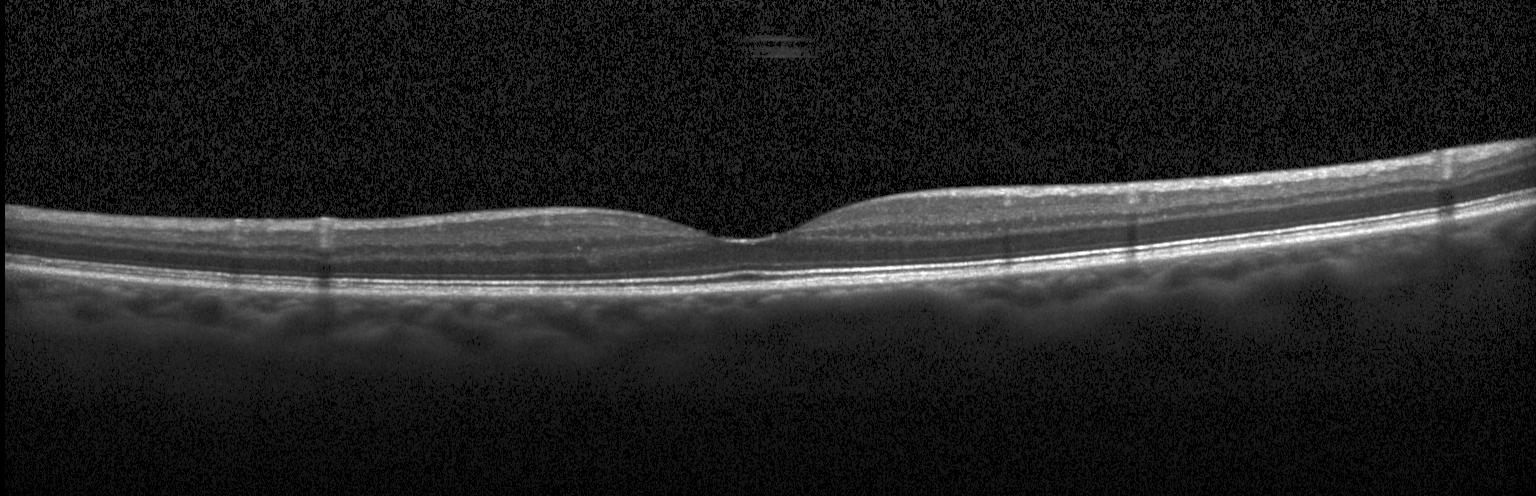
Finding: no evidence of choroidal neovascularization, diabetic macular edema, or drusen.